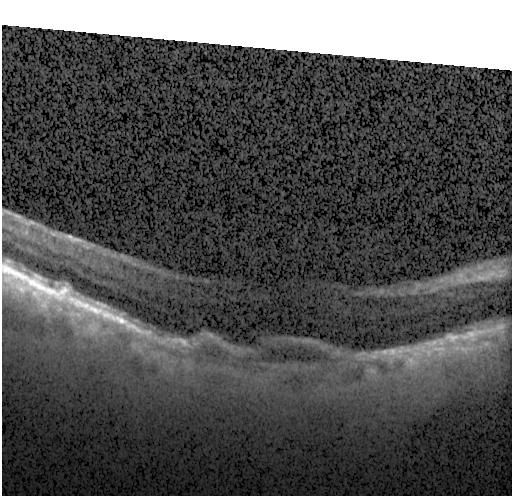
Macular OCT: a choroidal neovascular membrane.